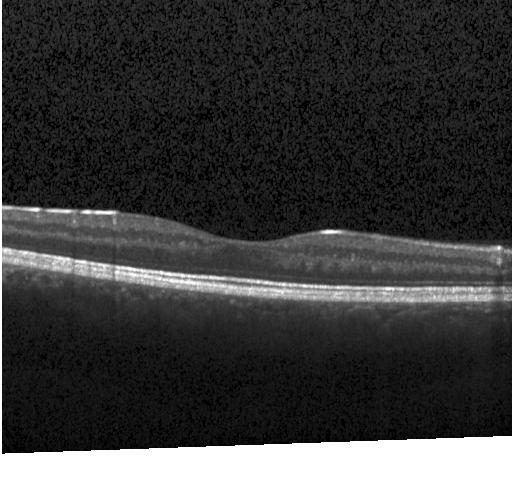 OCT scan showing neither CNV, DME, nor drusen.